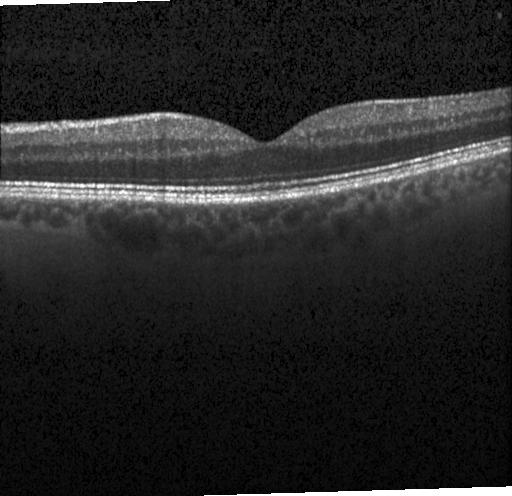

This B-scan demonstrates neither choroidal neovascularization, diabetic macular edema, nor drusen.